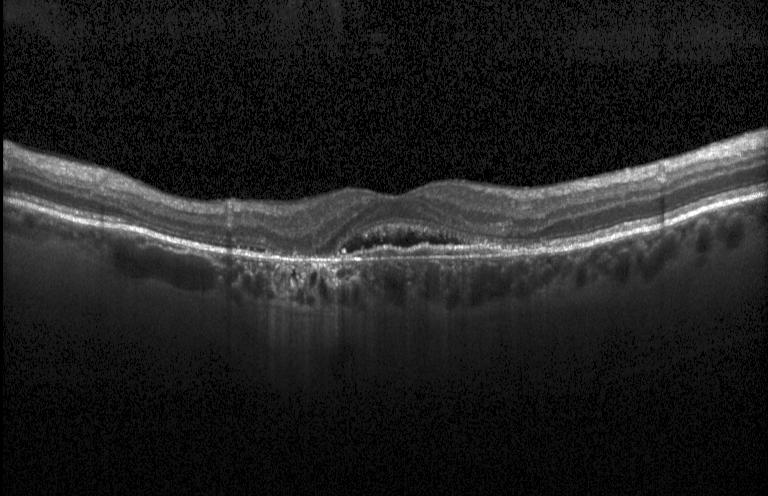

Macular OCT demonstrating choroidal neovascularization.